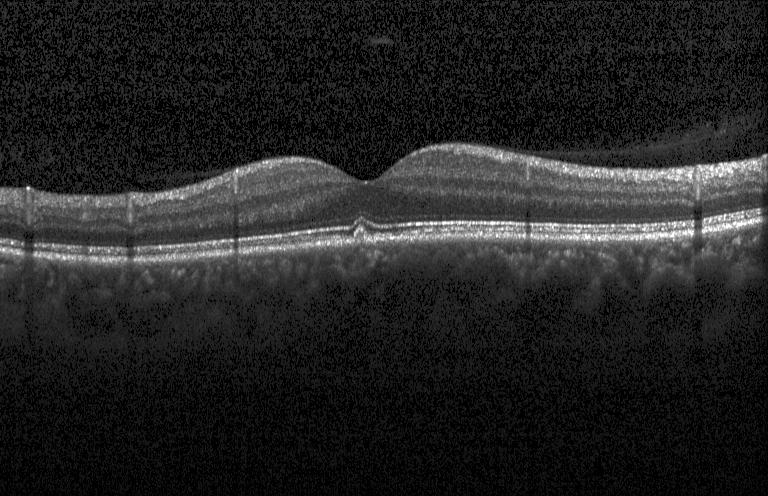 OCT B-scan — Multiple drusen.